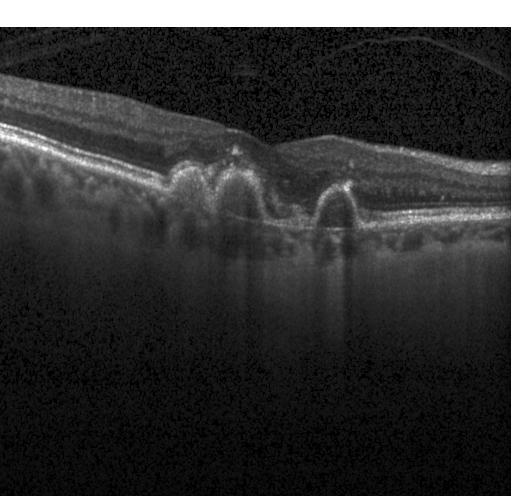 Finding: CNV.